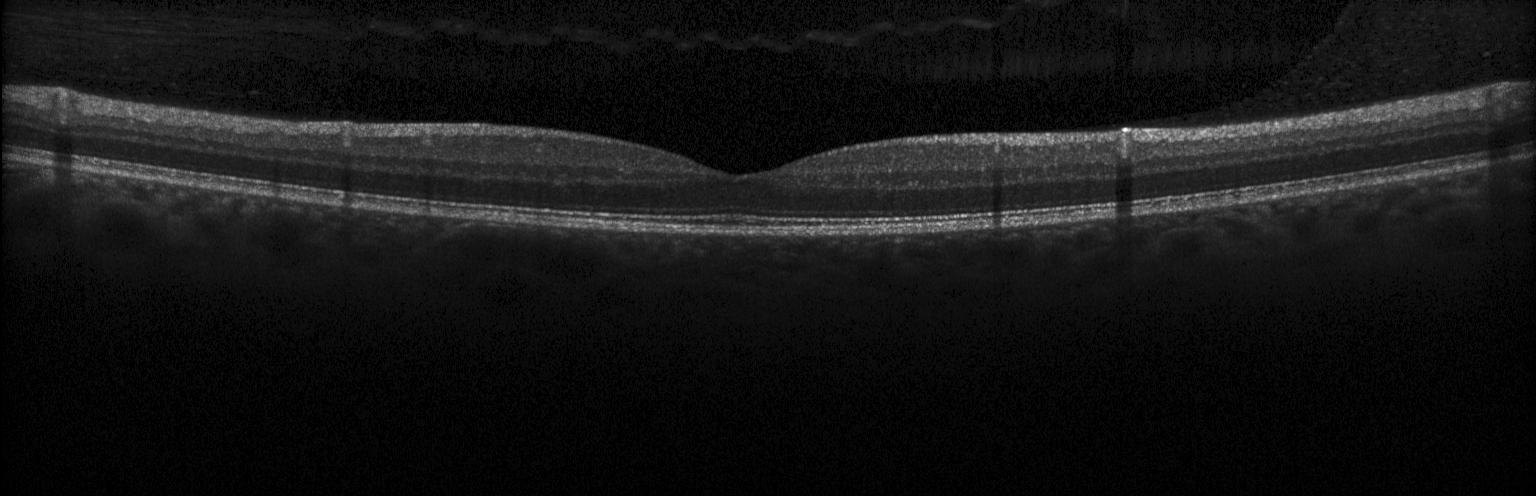 Diagnosis: no choroidal neovascularization, no diabetic macular edema, and no drusen.